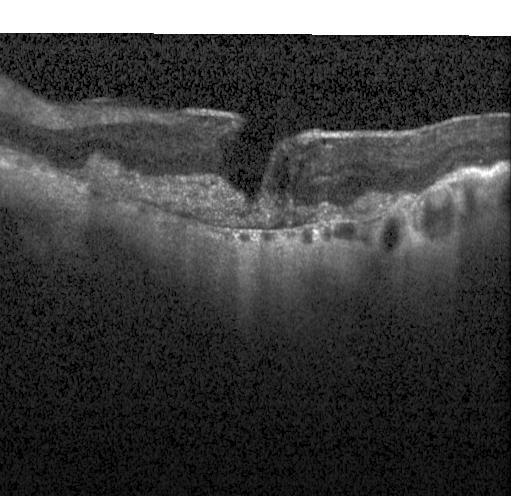
Macular OCT: CNV.